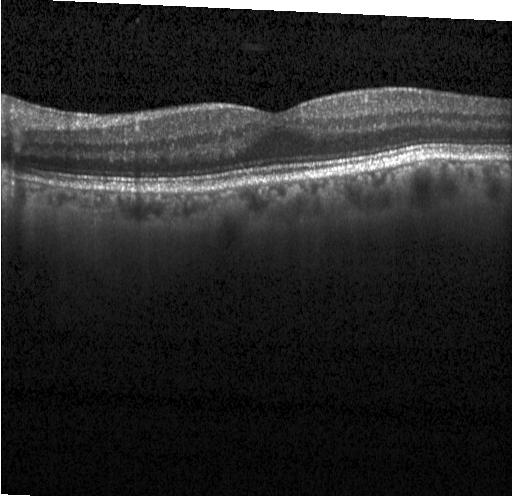 Spectral-domain OCT B-scan: neither choroidal neovascularization, diabetic macular edema, nor drusen.